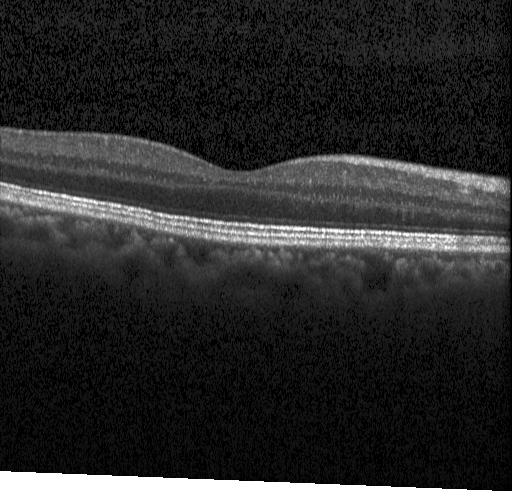

SD-OCT. Heidelberg Spectralis OCT system. Retinal OCT B-scan — The scan shows no CNV, DME, or drusen.